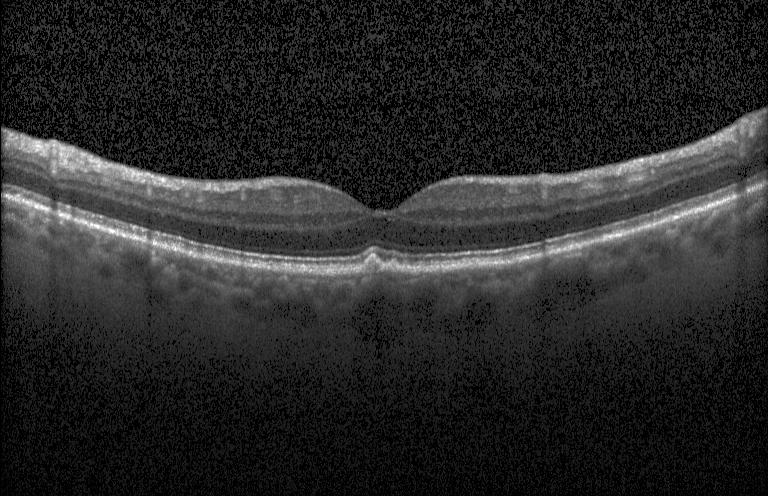

Acquired on a Heidelberg Spectralis; macular scan; retinal OCT cross-section.
The scan shows multiple drusen.